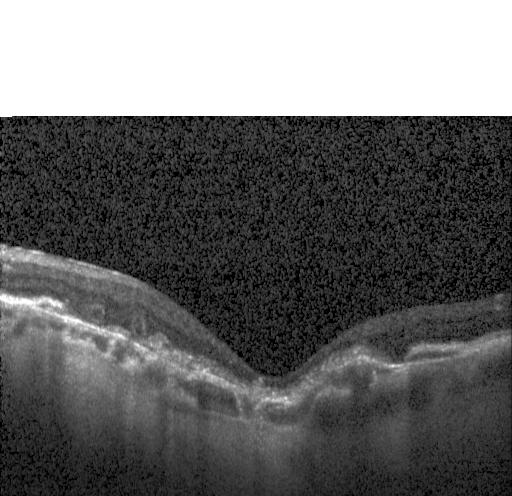
Macular scan; OCT B-scan; Heidelberg Spectralis OCT system — Finding: a choroidal neovascular membrane.